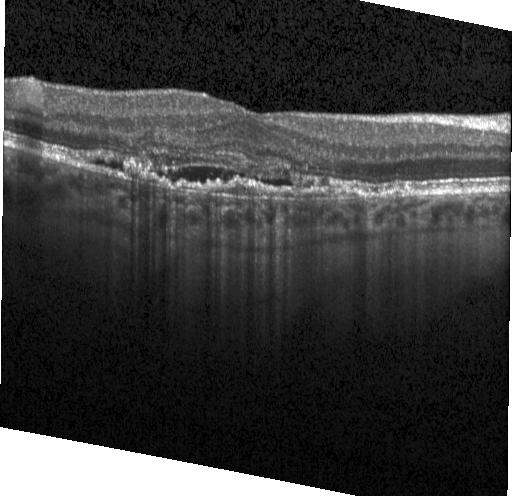 Optical coherence tomography B-scan. The scan shows choroidal neovascularization.